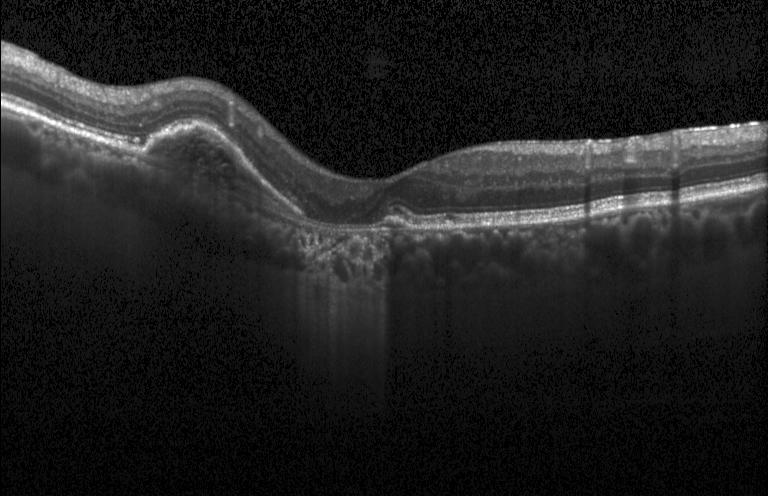
OCT B-scan
Assessment: CNV.